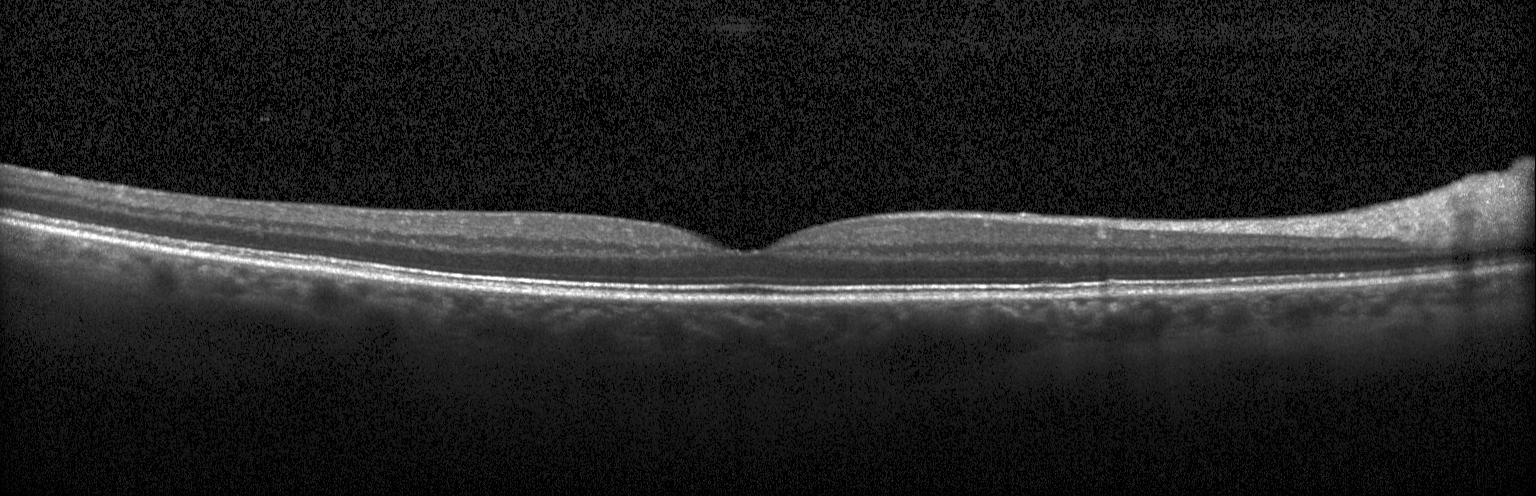
Retinal OCT cross-section, Heidelberg Spectralis
Dx: no evidence of choroidal neovascularization, diabetic macular edema, or drusen.